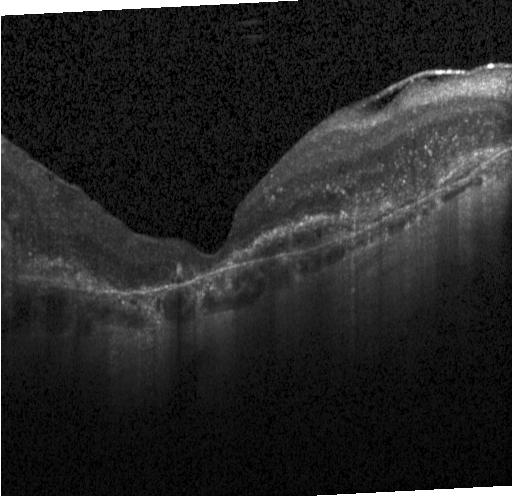 Optical coherence tomography scan. Spectral-domain OCT
Diagnosis: a choroidal neovascular membrane.